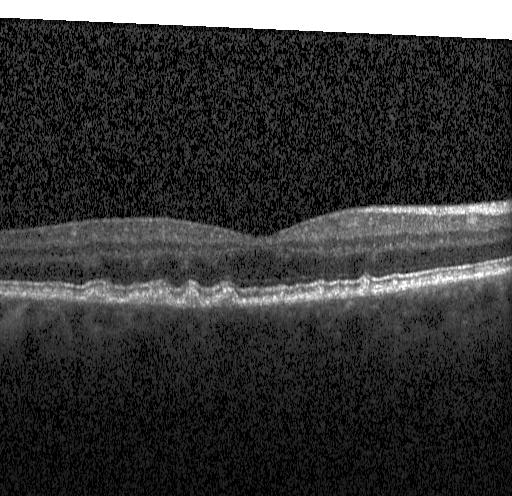 Fovea-centered, OCT line scan. Impression: multiple drusen.